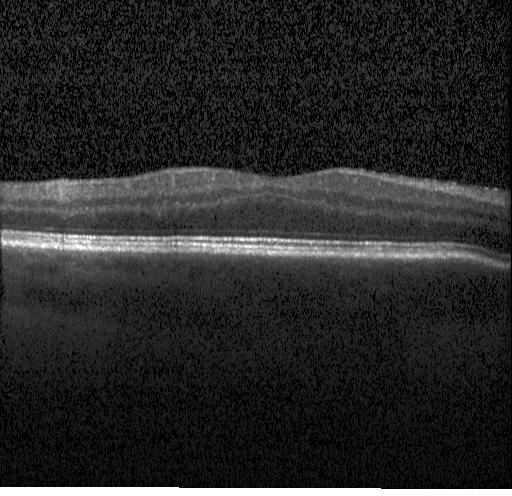

Optical coherence tomography scan. Spectral-domain OCT. Acquired on a Heidelberg Spectralis. Finding: no evidence of choroidal neovascularization, diabetic macular edema, or drusen.